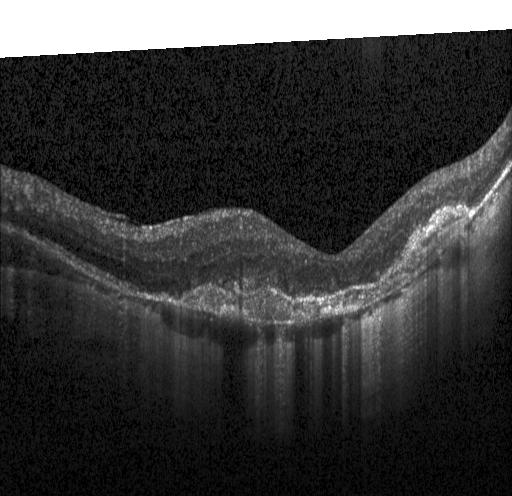

OCT B-scan · spectral-domain optical coherence tomography. Dx: choroidal neovascularization.